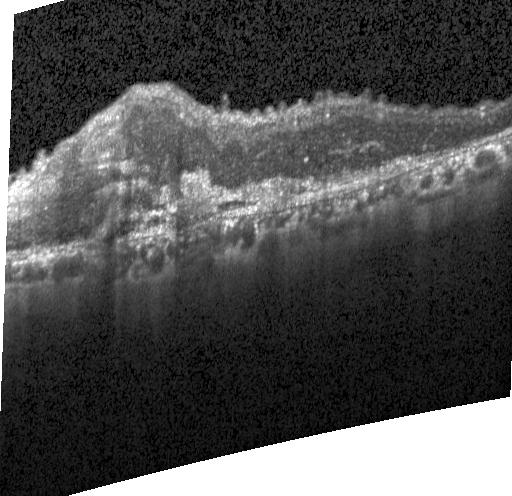 The scan shows a choroidal neovascular membrane.